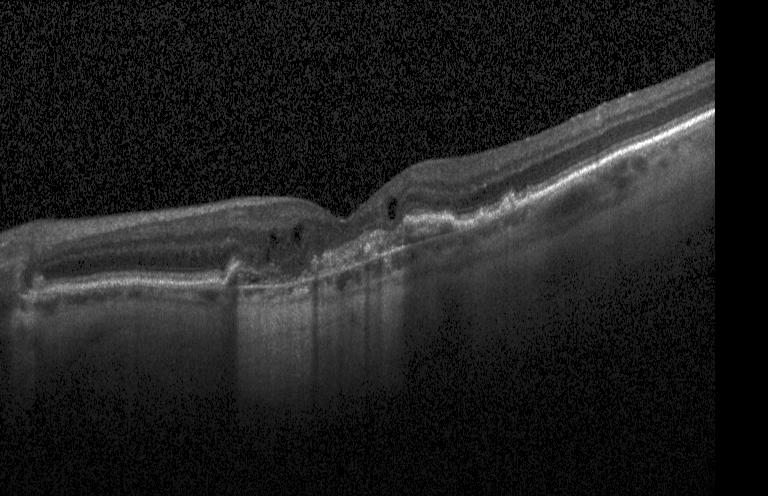

Macular OCT: CNV.